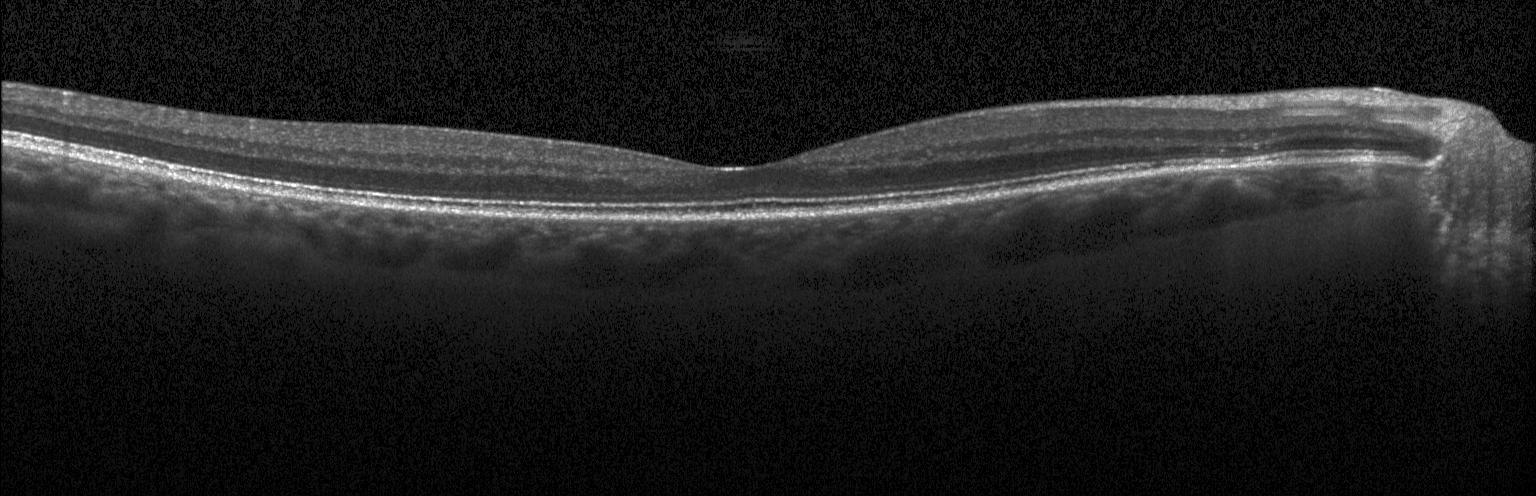

Heidelberg Spectralis OCT system; OCT line scan.
OCT finding: no evidence of CNV, DME, or drusen.